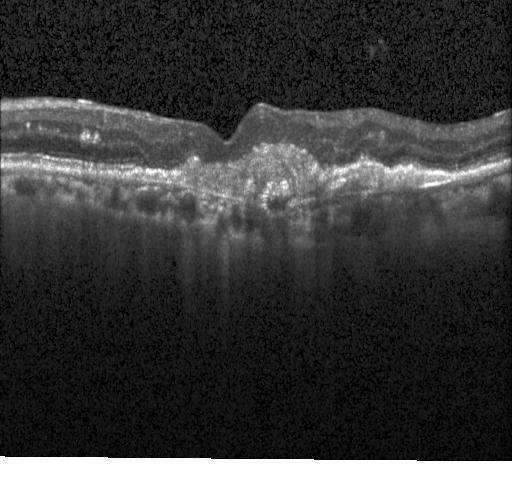
OCT scan showing CNV.